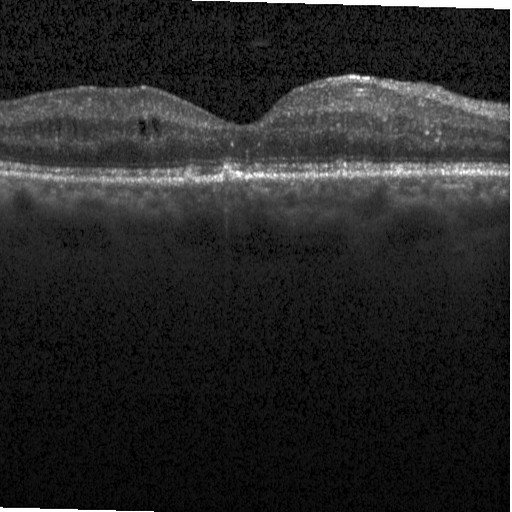

Assessment: diabetic macular edema (DME).